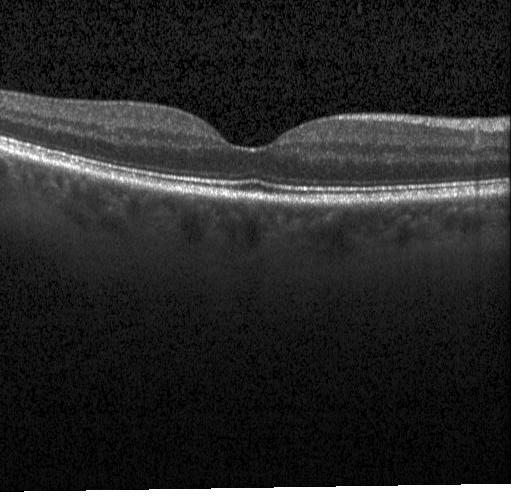 Assessment: no choroidal neovascularization, diabetic macular edema, or drusen.